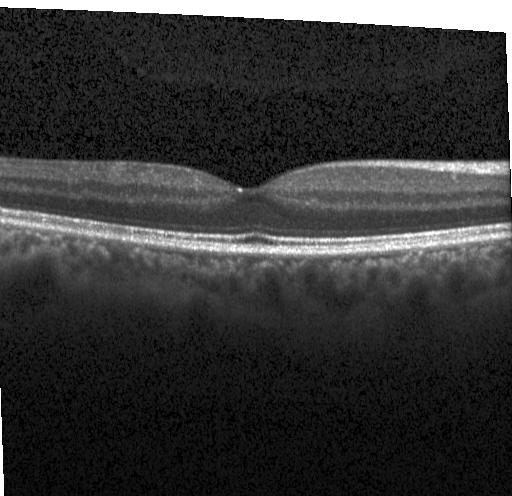

Spectral-domain OCT. Optical coherence tomography scan. Macular scan. Heidelberg Spectralis — Dx: no choroidal neovascularization, no diabetic macular edema, and no drusen.